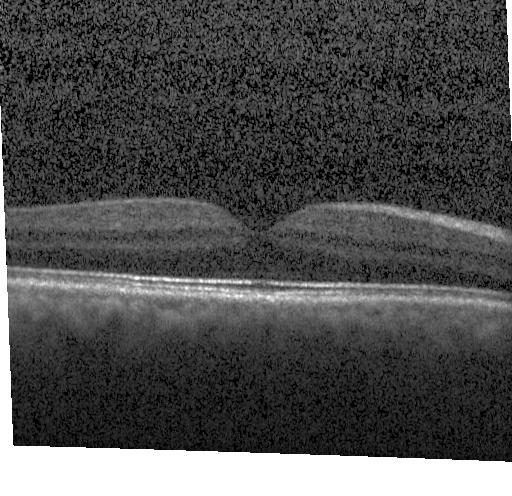

OCT line scan · Heidelberg Spectralis OCT system · macular scan — Impression: no CNV, DME, or drusen.